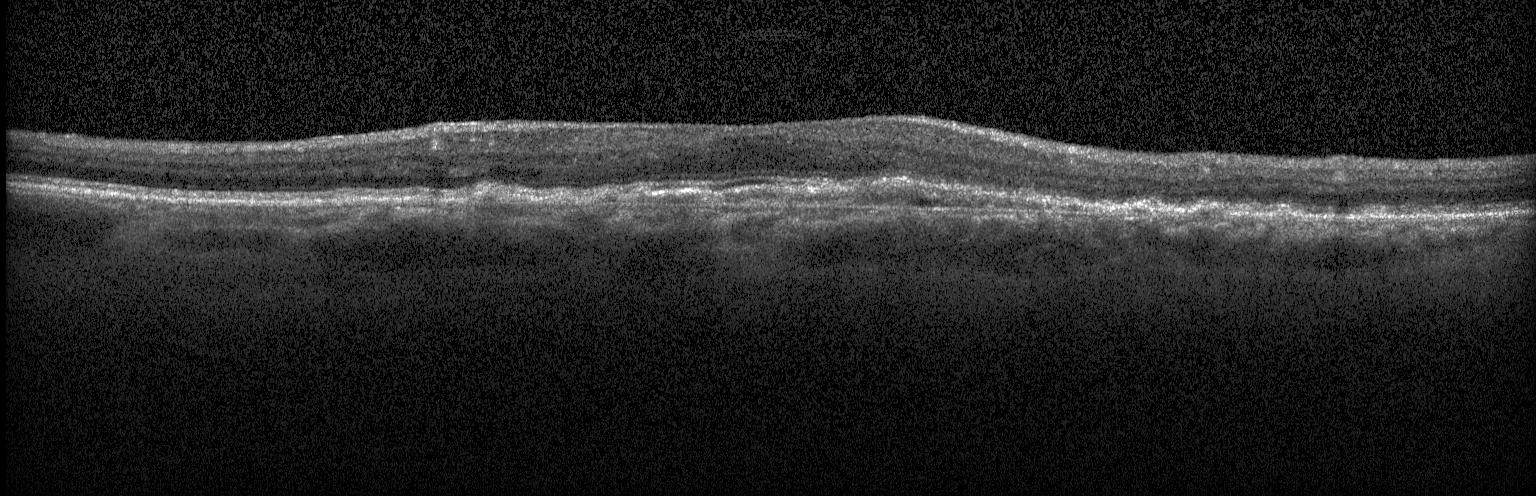

Through the macula · spectral-domain optical coherence tomography · OCT B-scan
Finding: choroidal neovascularization (CNV).